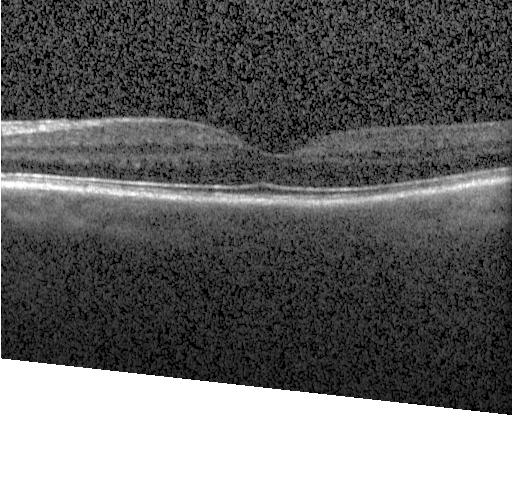
The scan shows no evidence of choroidal neovascularization, diabetic macular edema, or drusen.